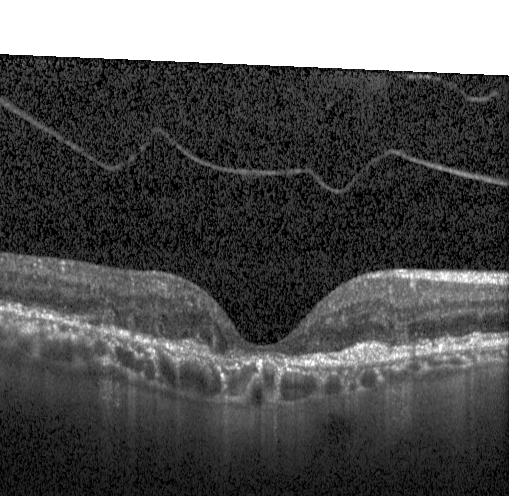 Retinal OCT B-scan · through the macula · Heidelberg Spectralis OCT system
Impression: a choroidal neovascular membrane.